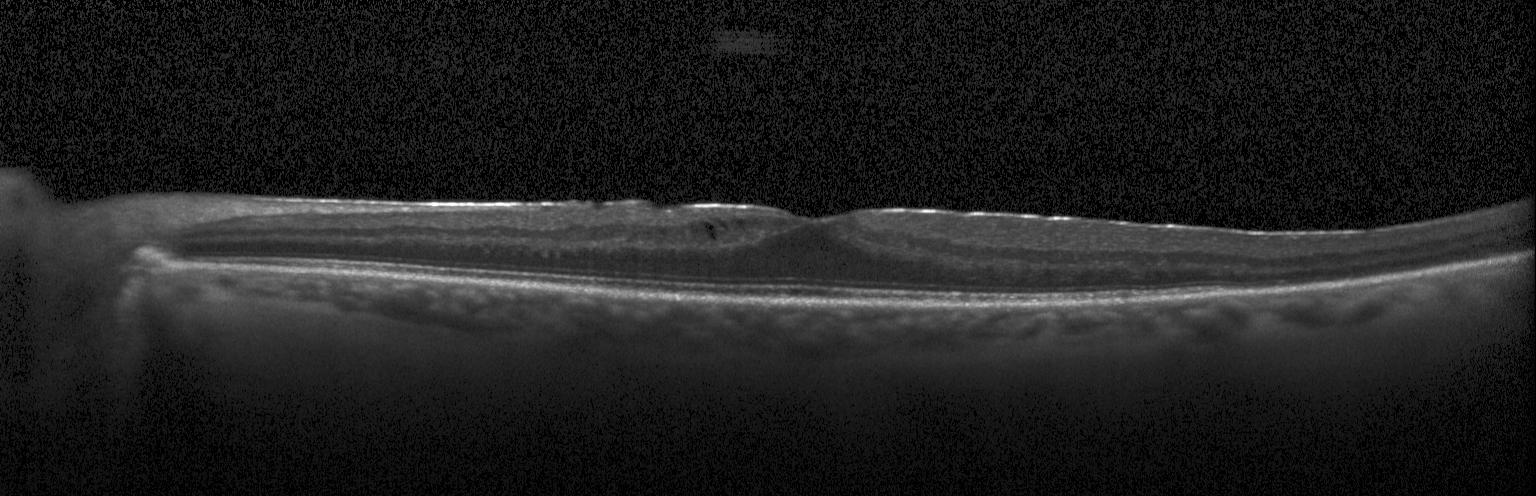
Macular OCT: DME.